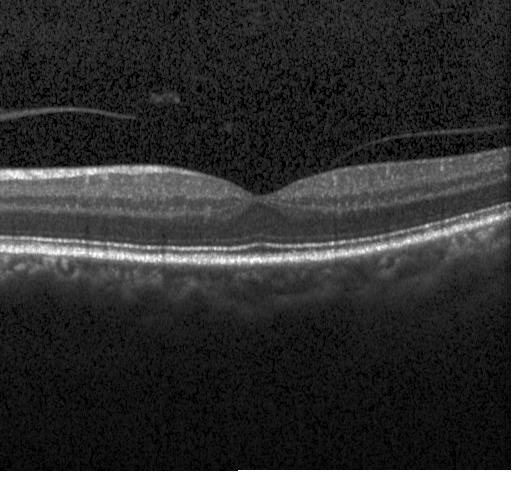

Retinal OCT B-scan · acquired on a Heidelberg Spectralis — Dx: no choroidal neovascularization, diabetic macular edema, or drusen.